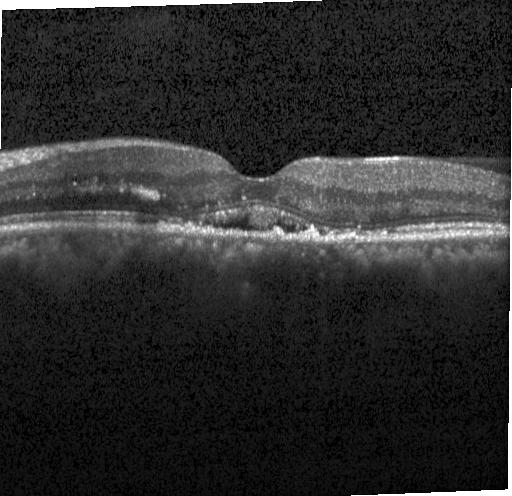
A choroidal neovascular membrane.